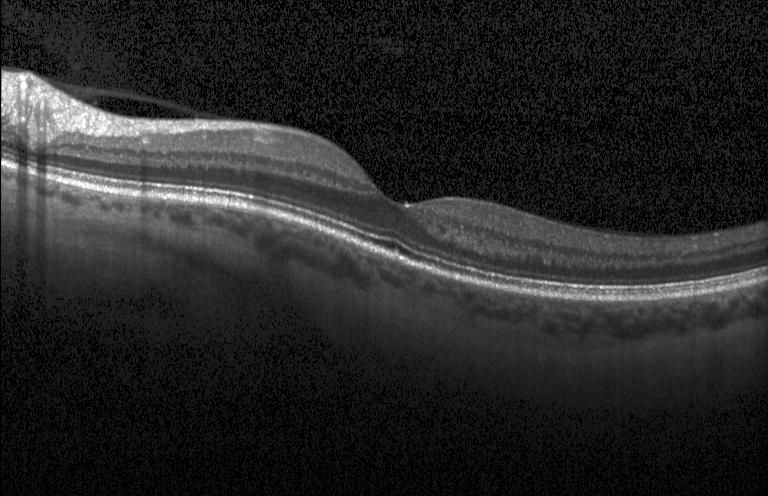

The scan shows no evidence of CNV, DME, or drusen.